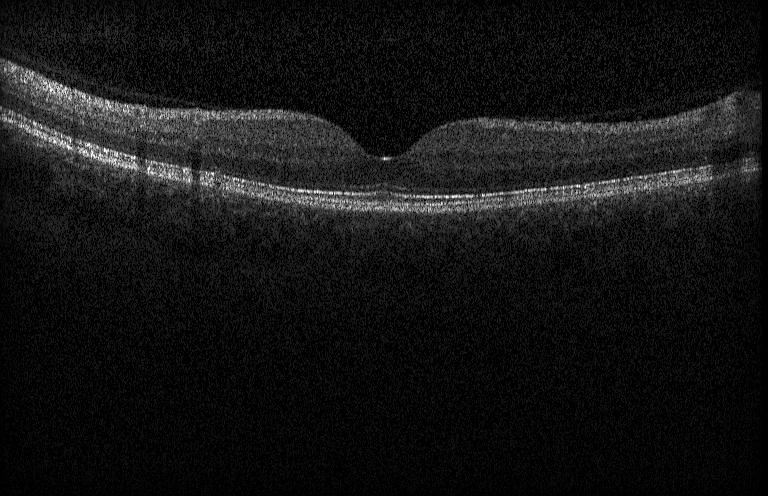

Heidelberg Spectralis OCT system · retinal OCT B-scan · centered on the fovea
Finding: neither choroidal neovascularization, diabetic macular edema, nor drusen.